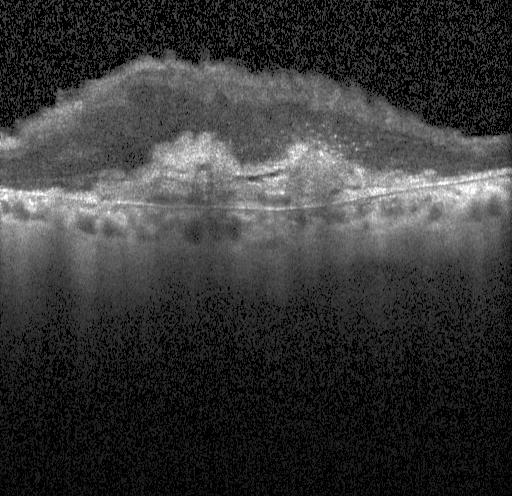 Impression: a choroidal neovascular membrane.